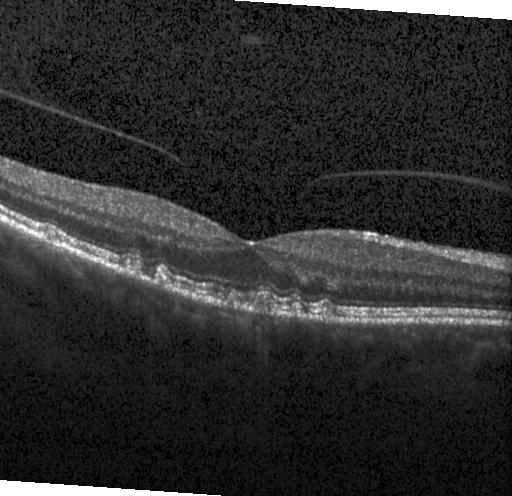 Spectral-domain optical coherence tomography; acquired on a Heidelberg Spectralis; optical coherence tomography B-scan
Finding: drusen.